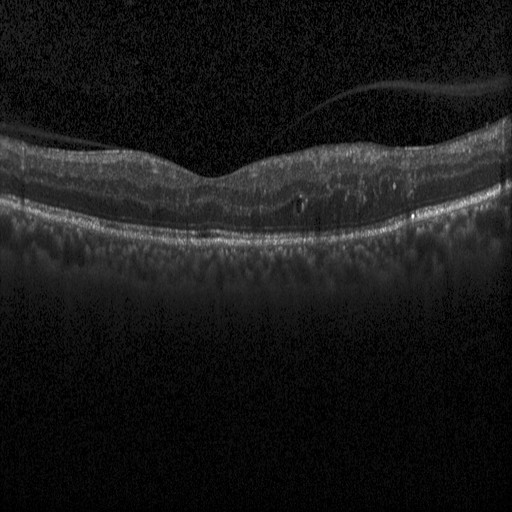

Impression: DME.